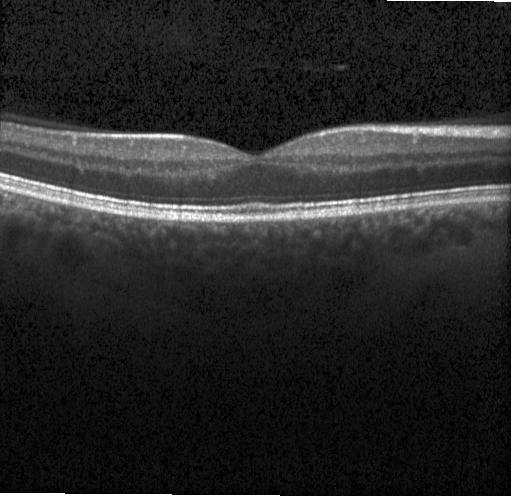 OCT B-scan; acquired on a Heidelberg Spectralis; through the macula
Finding: no evidence of choroidal neovascularization, diabetic macular edema, or drusen.